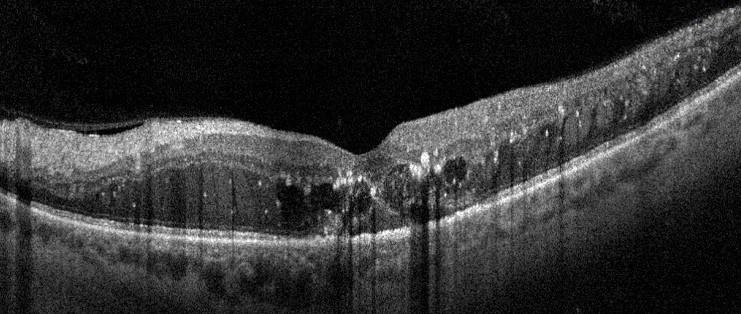 Optovue Avanti RTVue XR; retinal OCT cross-section
Impression: DME.